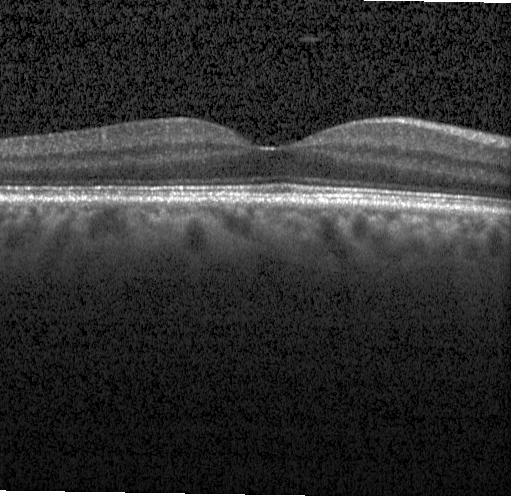
Heidelberg Spectralis OCT system · optical coherence tomography B-scan.
Impression: no CNV, no DME, and no drusen.